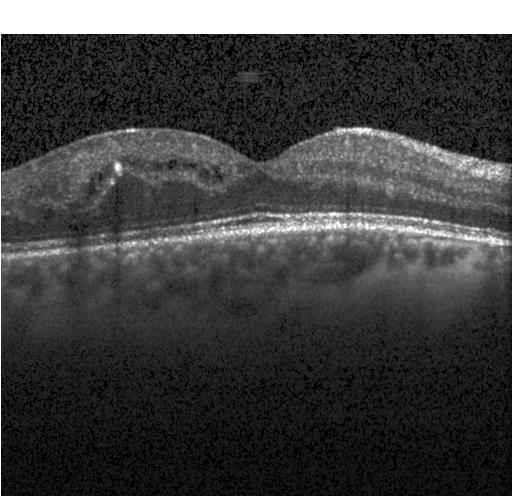
Retinal OCT cross-section.
Dx: diabetic macular edema.